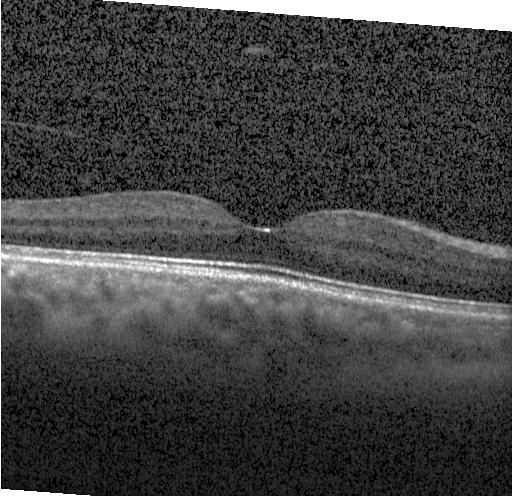
Centered on the fovea; instrument: Heidelberg Spectralis; spectral-domain OCT; OCT B-scan.
Impression: no choroidal neovascularization, diabetic macular edema, or drusen.